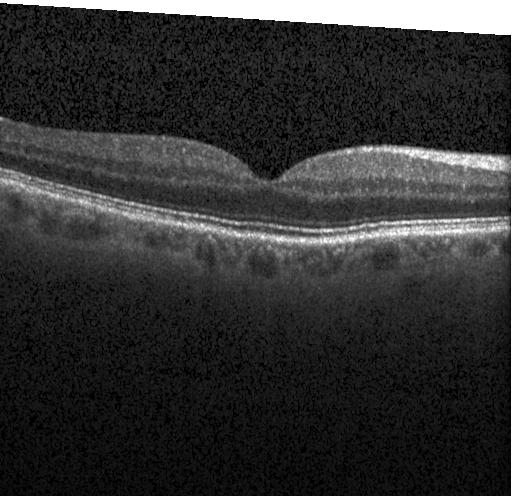

Retinal OCT cross-section; spectral-domain optical coherence tomography — OCT finding: no evidence of choroidal neovascularization, diabetic macular edema, or drusen.